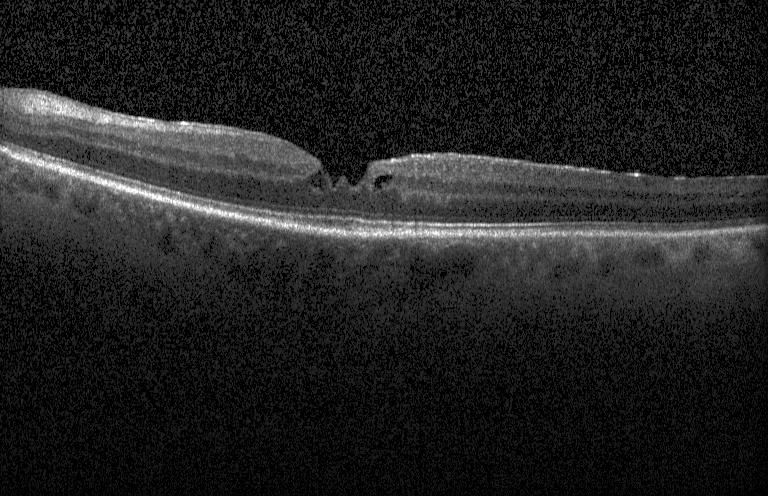

OCT finding: diabetic macular edema (DME).